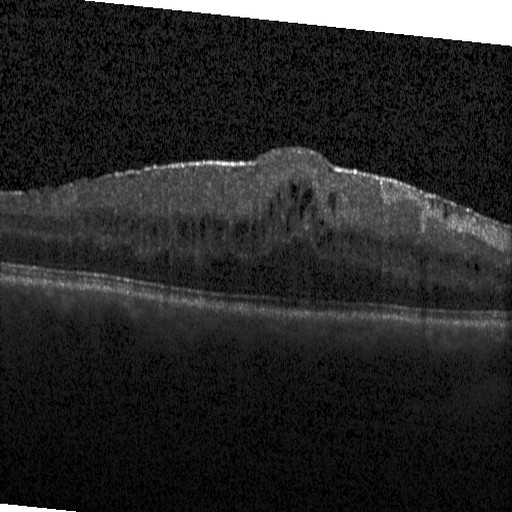

OCT finding: diabetic macular edema.